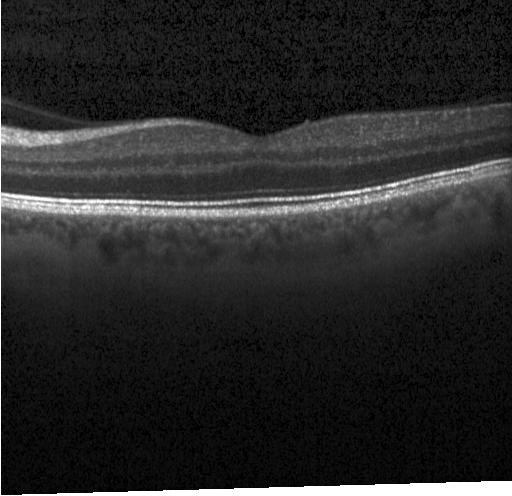 Macular OCT: neither CNV, DME, nor drusen.